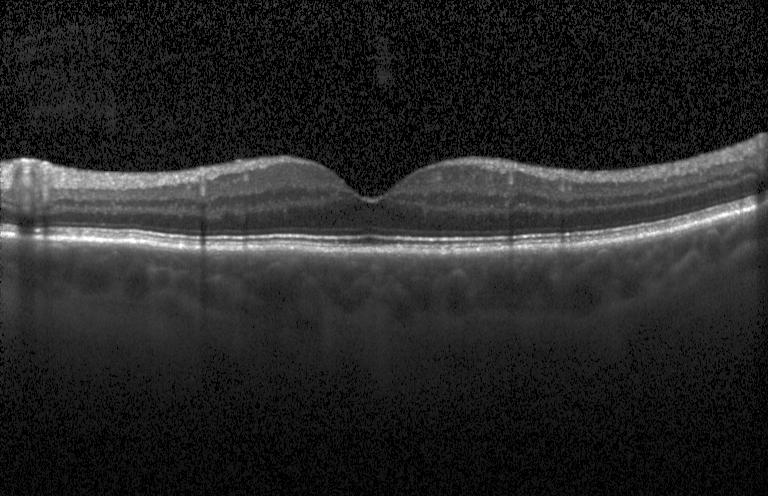 OCT B-scan showing no evidence of choroidal neovascularization, diabetic macular edema, or drusen.